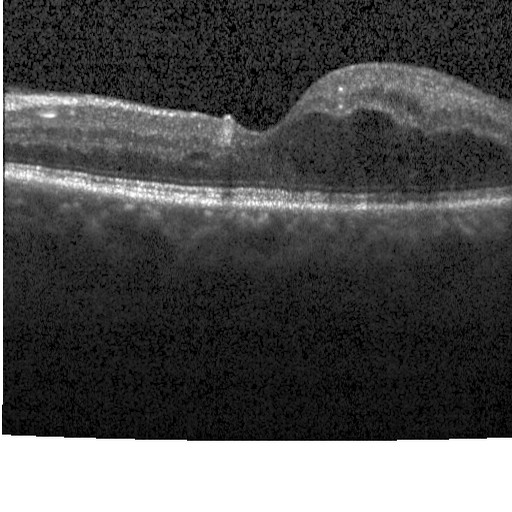 Macular scan; retinal OCT B-scan; instrument: Heidelberg Spectralis
Finding: diabetic macular edema (DME).